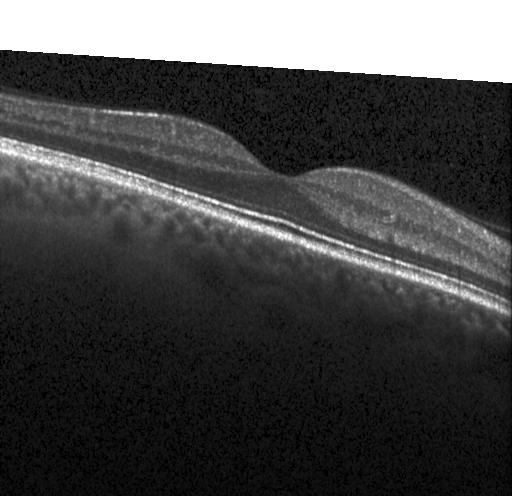

Finding: neither CNV, DME, nor drusen.